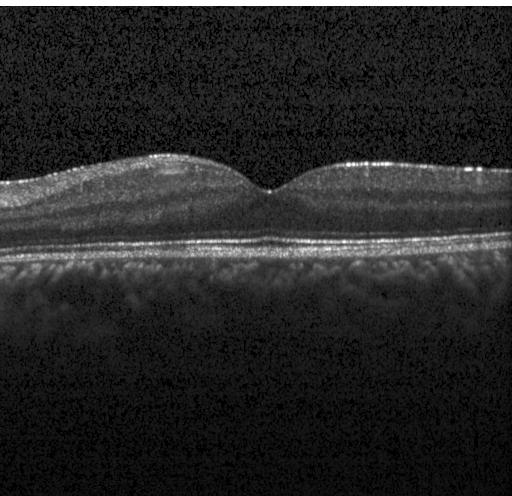

OCT line scan
Assessment: neither CNV, DME, nor drusen.